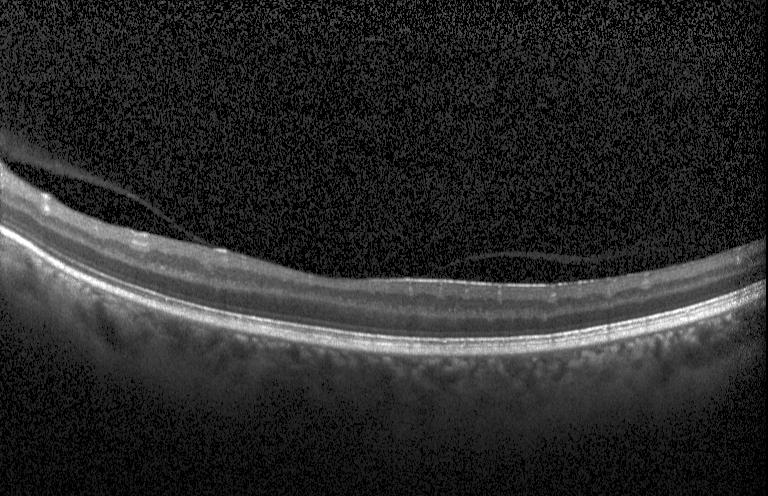
Spectral-domain OCT; OCT B-scan. Impression: neither choroidal neovascularization, diabetic macular edema, nor drusen.